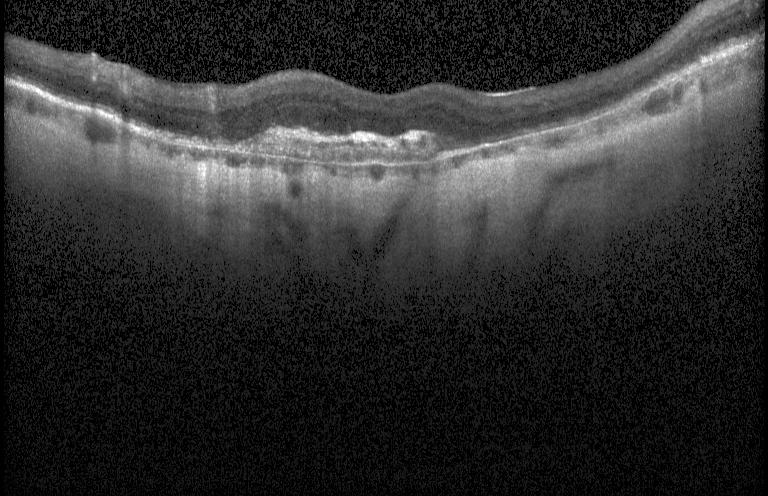

OCT line scan
Impression: choroidal neovascularization.